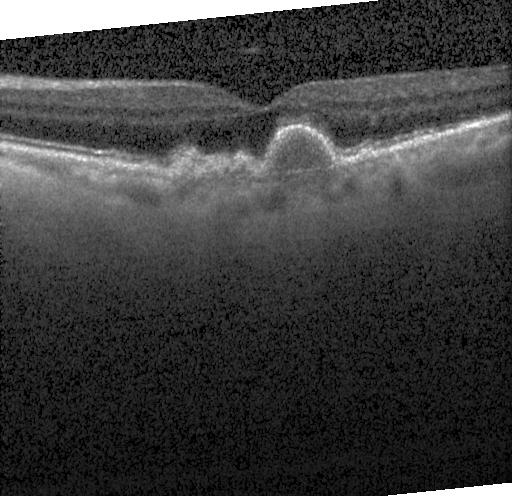
Retinal OCT cross-section.
Diagnosis: drusen.